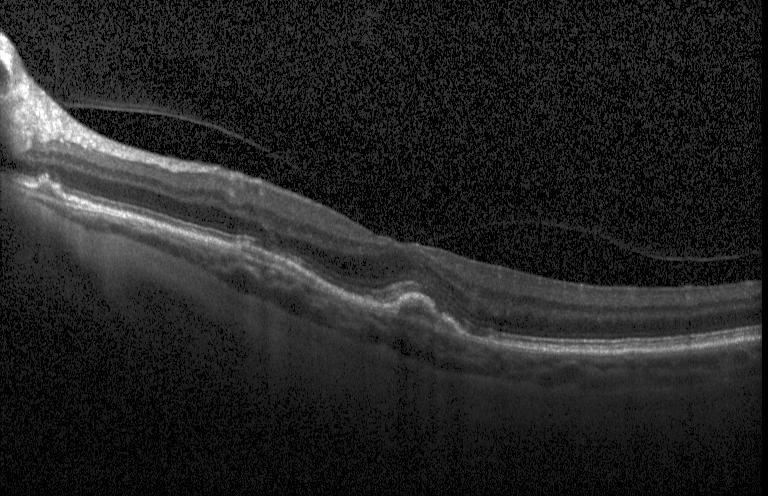
Diagnosis: sub-RPE drusenoid deposits.